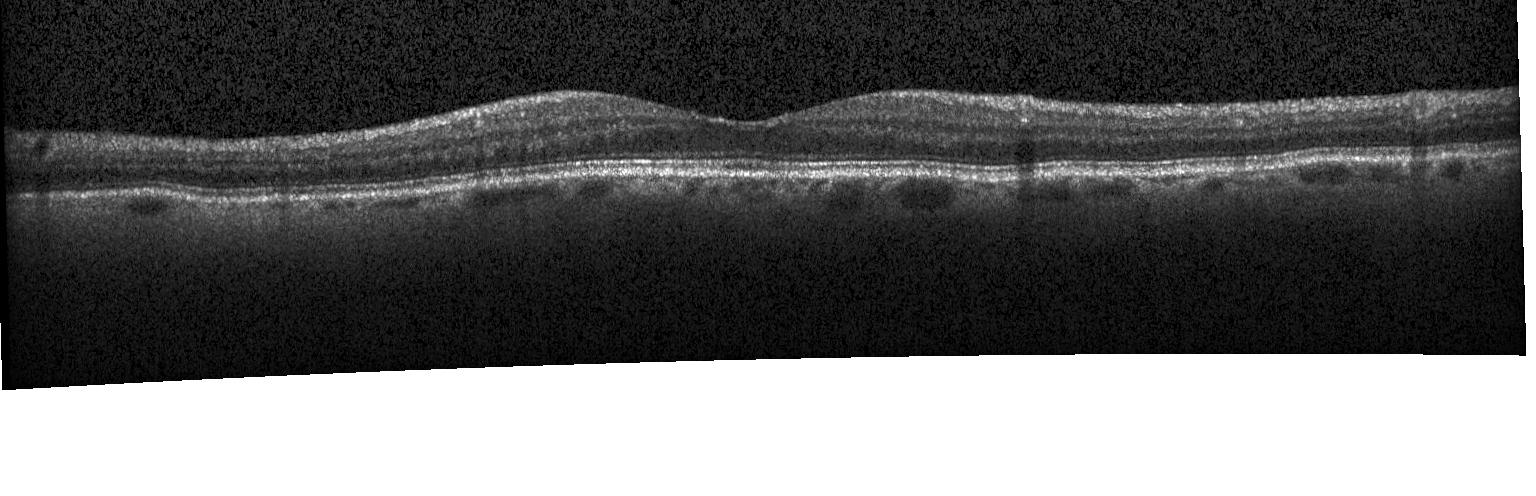
Centered on the fovea. Retinal OCT B-scan
Dx: neither choroidal neovascularization, diabetic macular edema, nor drusen.